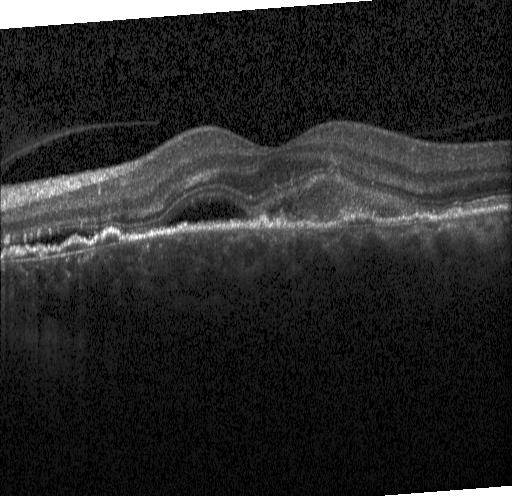 Spectral-domain optical coherence tomography. Through the macula. Optical coherence tomography scan. Acquired on a Heidelberg Spectralis — The scan shows CNV.